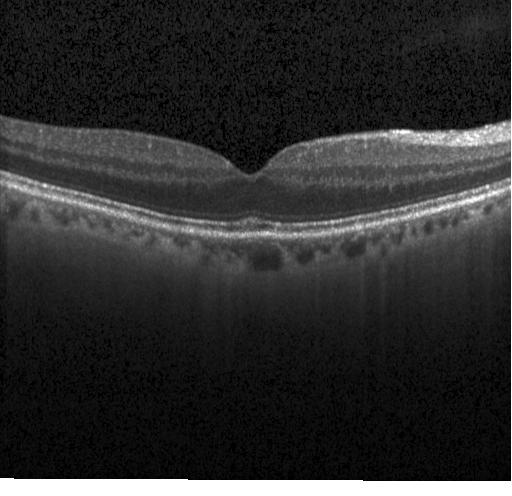

OCT line scan
Diagnosis: no evidence of choroidal neovascularization, diabetic macular edema, or drusen.